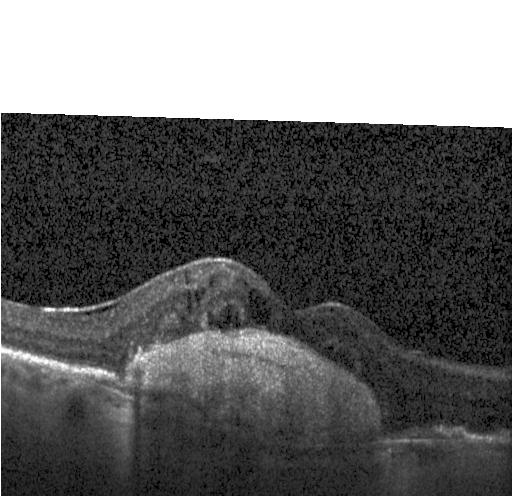

Macular scan; optical coherence tomography scan — This B-scan demonstrates a choroidal neovascular membrane.